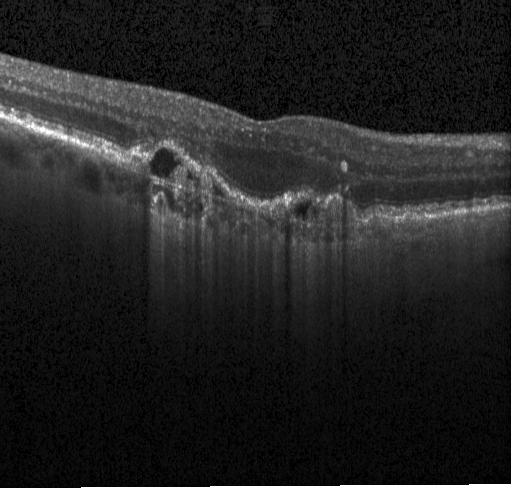
Diagnosis: a choroidal neovascular membrane.